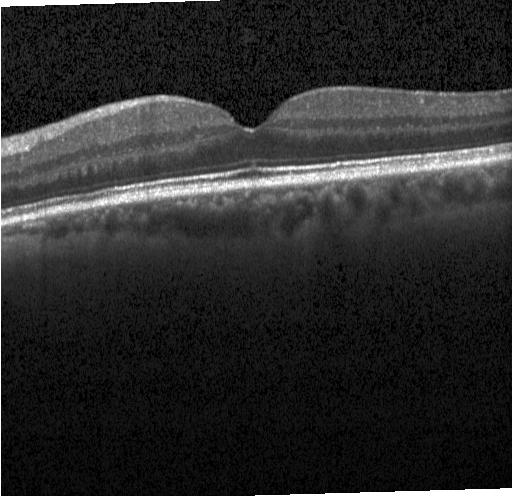

Retinal OCT cross-section. No evidence of choroidal neovascularization, diabetic macular edema, or drusen.